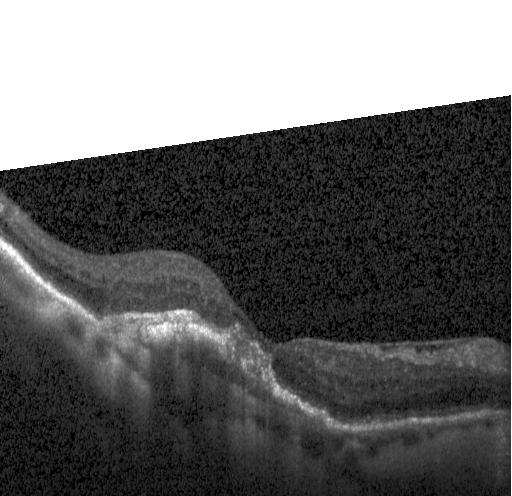
Retinal OCT cross-section — OCT finding: choroidal neovascularization (CNV).